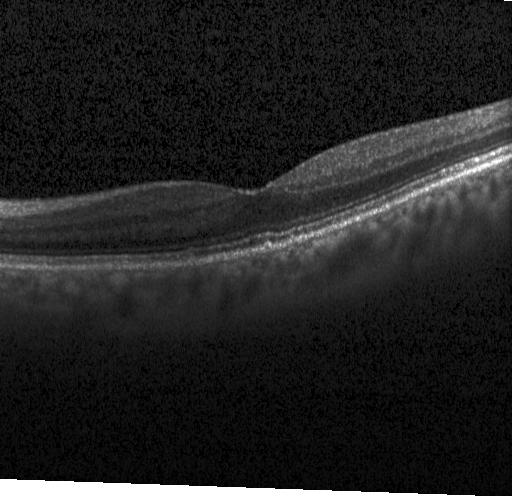 Diagnosis: multiple drusen.